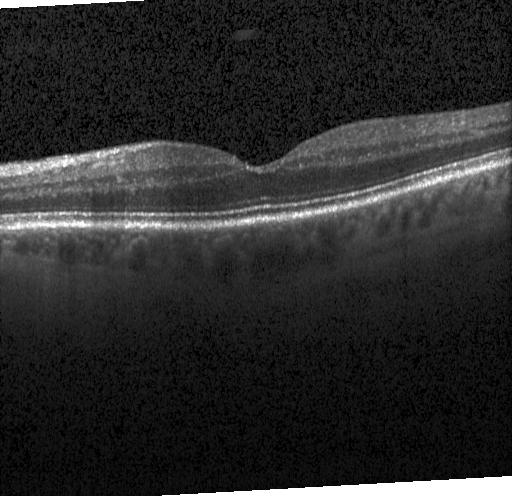 OCT B-scan; Heidelberg Spectralis; through the macula; SD-OCT
No choroidal neovascularization, no diabetic macular edema, and no drusen.